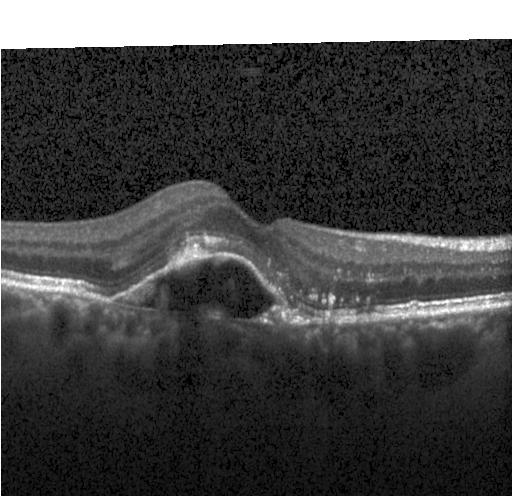
Spectral-domain OCT B-scan: a choroidal neovascular membrane.